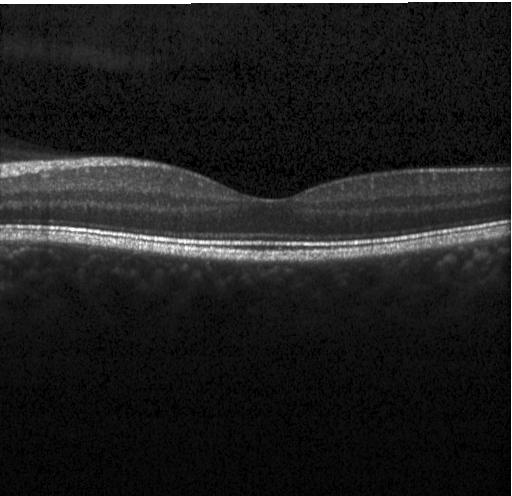

Heidelberg Spectralis. Fovea-centered. Spectral-domain OCT. Optical coherence tomography scan. The scan shows no choroidal neovascularization, no diabetic macular edema, and no drusen.